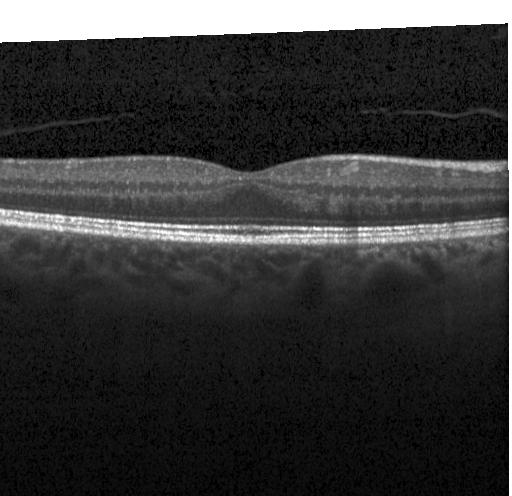
Instrument: Heidelberg Spectralis · centered on the fovea · retinal OCT cross-section.
Impression: no choroidal neovascularization, diabetic macular edema, or drusen.